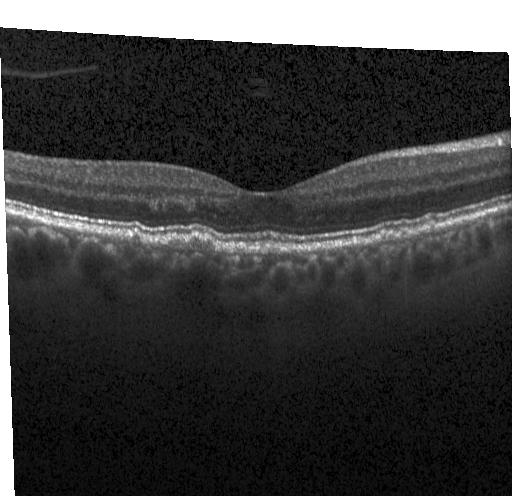
Retinal OCT cross-section. Finding: sub-RPE drusenoid deposits.